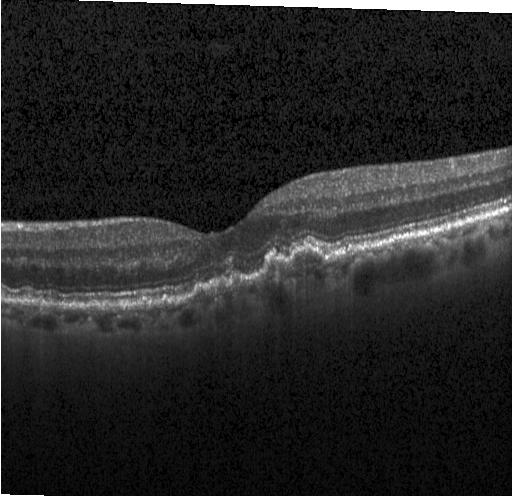

Multiple drusen.